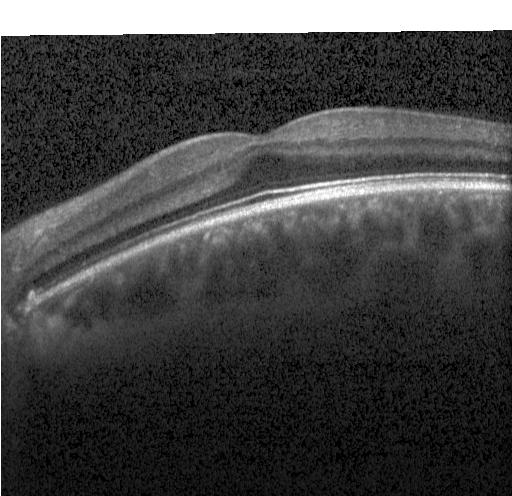 Dx: no evidence of choroidal neovascularization, diabetic macular edema, or drusen.